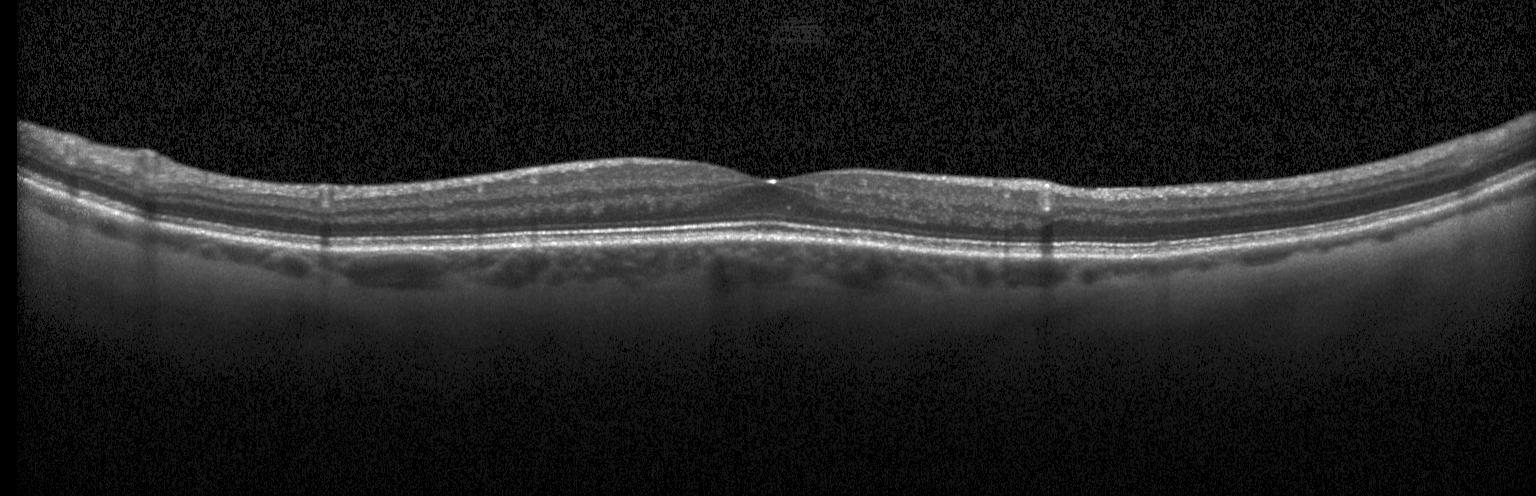

Spectral-domain OCT B-scan: no CNV, no DME, and no drusen.